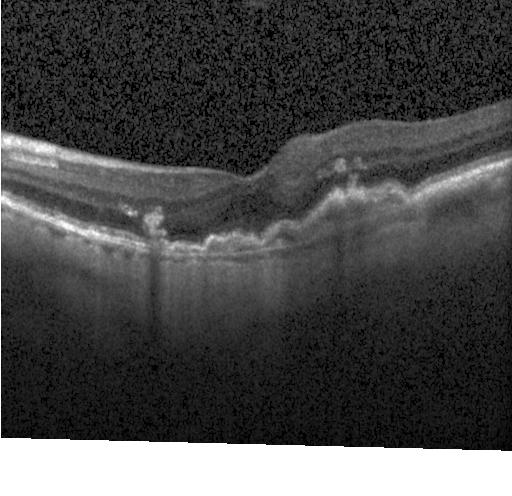

Optical coherence tomography scan.
Finding: a choroidal neovascular membrane.